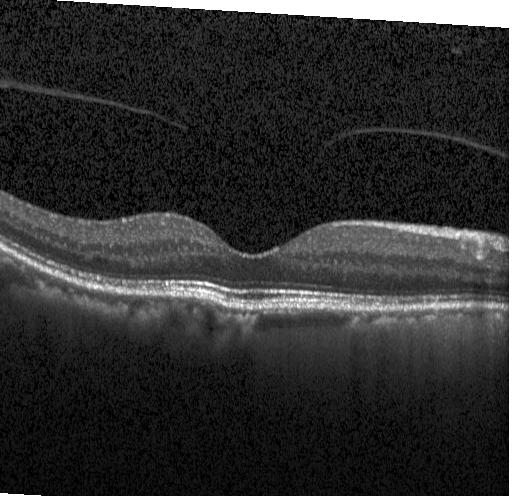 Instrument: Heidelberg Spectralis · SD-OCT · OCT B-scan · through the macula.
No CNV, no DME, and no drusen.